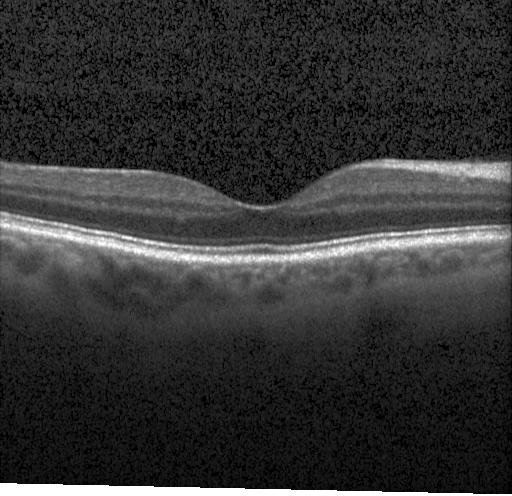 OCT finding: no evidence of choroidal neovascularization, diabetic macular edema, or drusen.